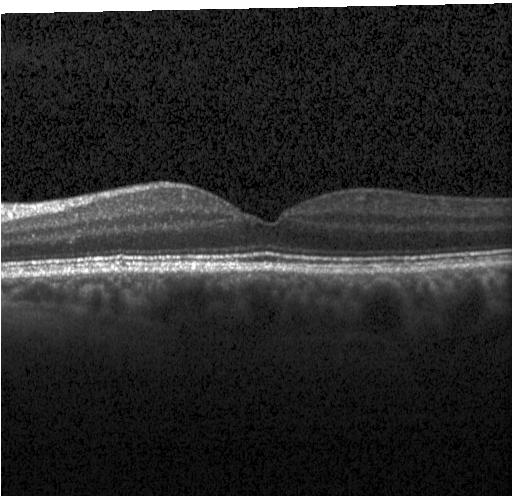 Retinal OCT cross-section. Diagnosis: neither choroidal neovascularization, diabetic macular edema, nor drusen.